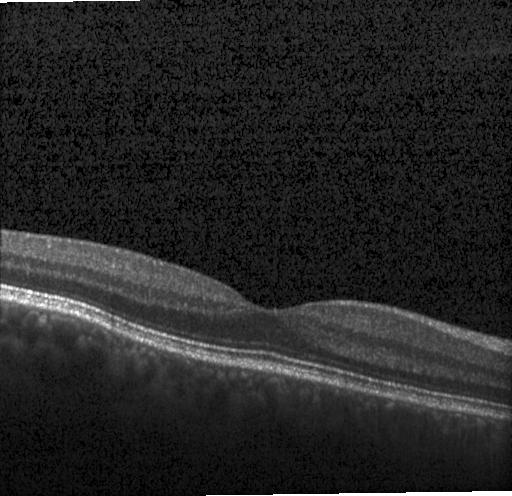 Through the macula · retinal OCT B-scan · Heidelberg Spectralis · SD-OCT.
Impression: no choroidal neovascularization, diabetic macular edema, or drusen.